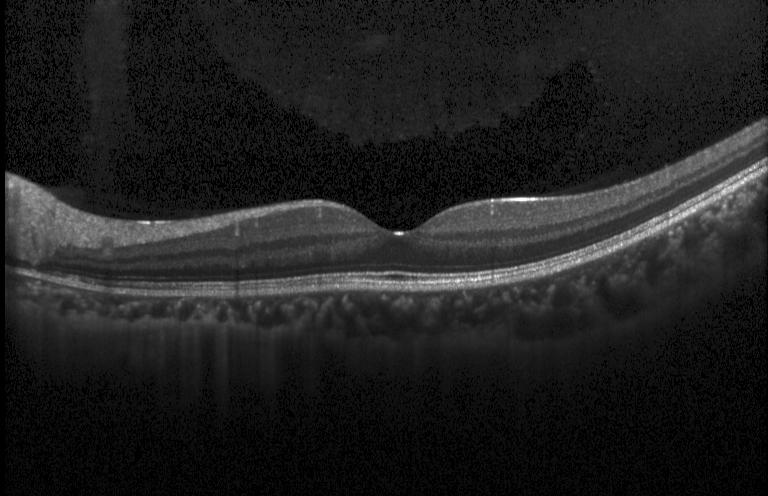
SD-OCT · OCT B-scan
Impression: no evidence of CNV, DME, or drusen.